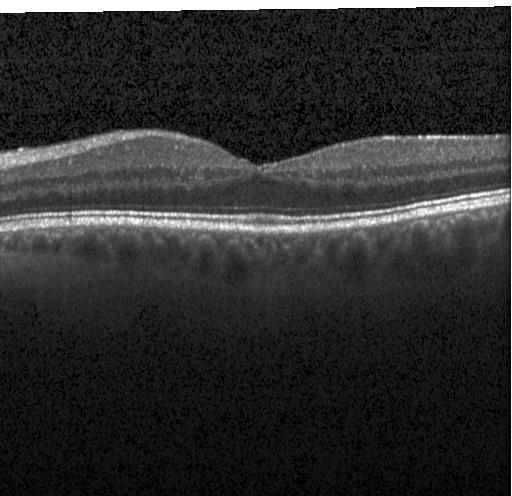
Diagnosis: neither choroidal neovascularization, diabetic macular edema, nor drusen.